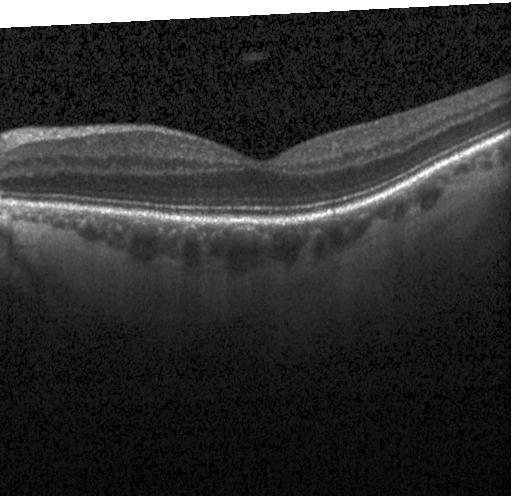 Retinal OCT cross-section showing no CNV, no DME, and no drusen.